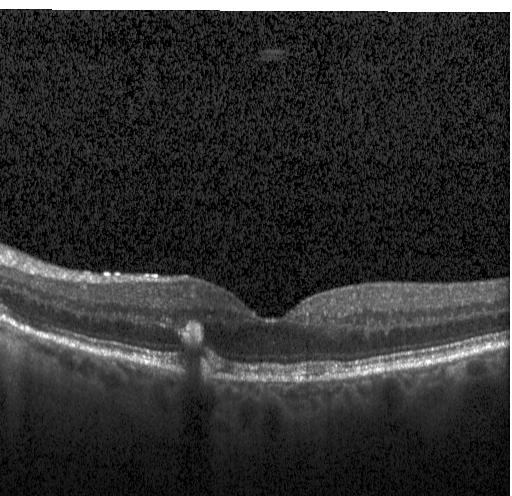
Optical coherence tomography B-scan · centered on the fovea · spectral-domain optical coherence tomography · acquired on a Heidelberg Spectralis.
Multiple drusen.